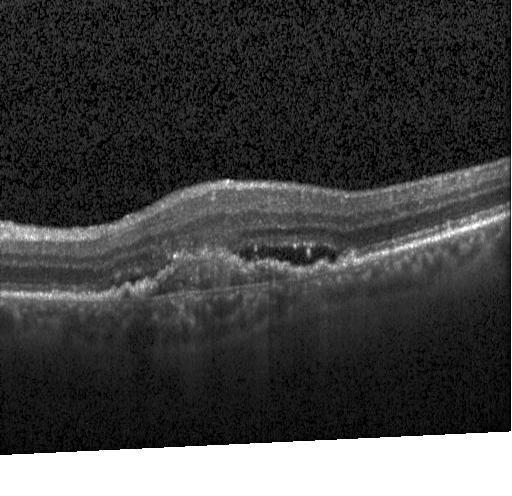
Retinal OCT B-scan · macular scan · instrument: Heidelberg Spectralis — Choroidal neovascularization.